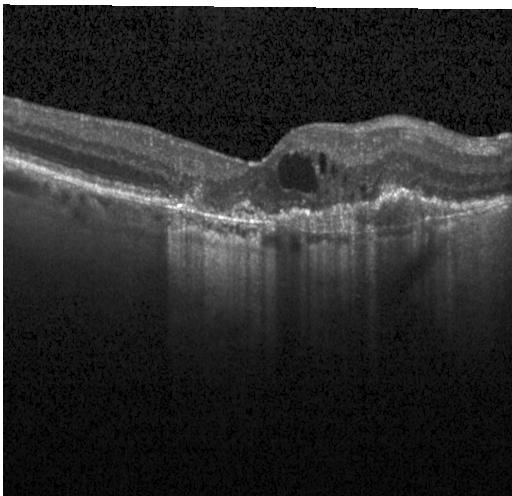
Impression: choroidal neovascularization (CNV).